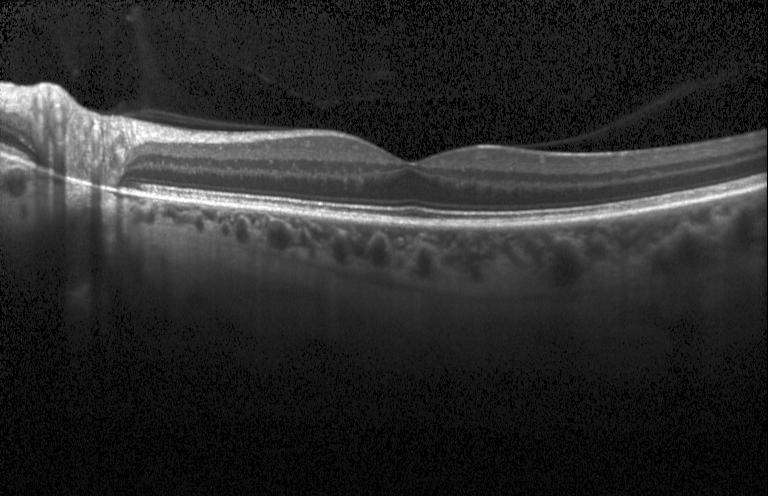 Heidelberg Spectralis OCT system; retinal OCT B-scan.
Diagnosis: neither choroidal neovascularization, diabetic macular edema, nor drusen.